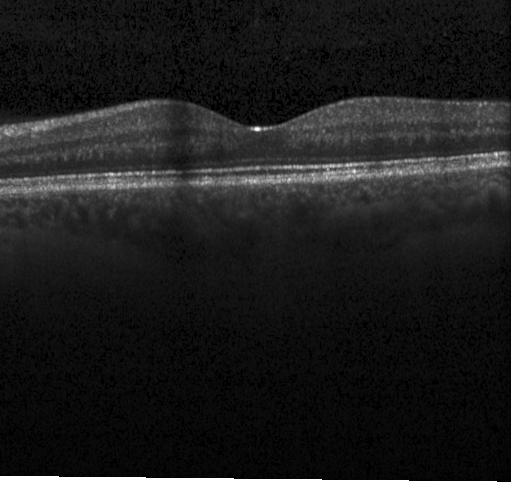 Through the macula. OCT B-scan — Dx: no evidence of choroidal neovascularization, diabetic macular edema, or drusen.